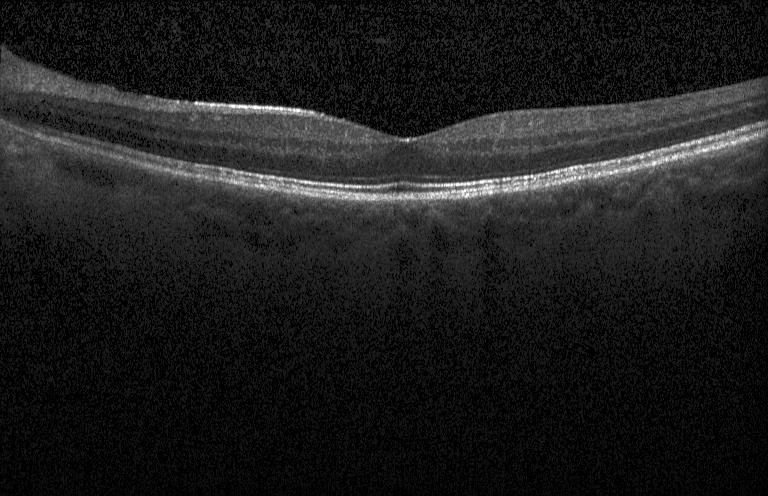

Heidelberg Spectralis, fovea-centered, optical coherence tomography scan.
No evidence of choroidal neovascularization, diabetic macular edema, or drusen.